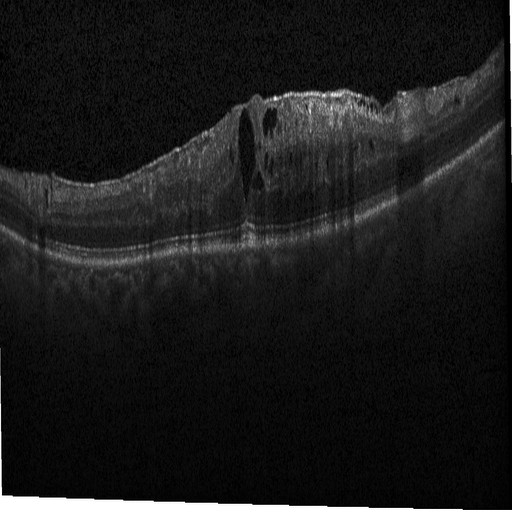
OCT B-scan. DME.